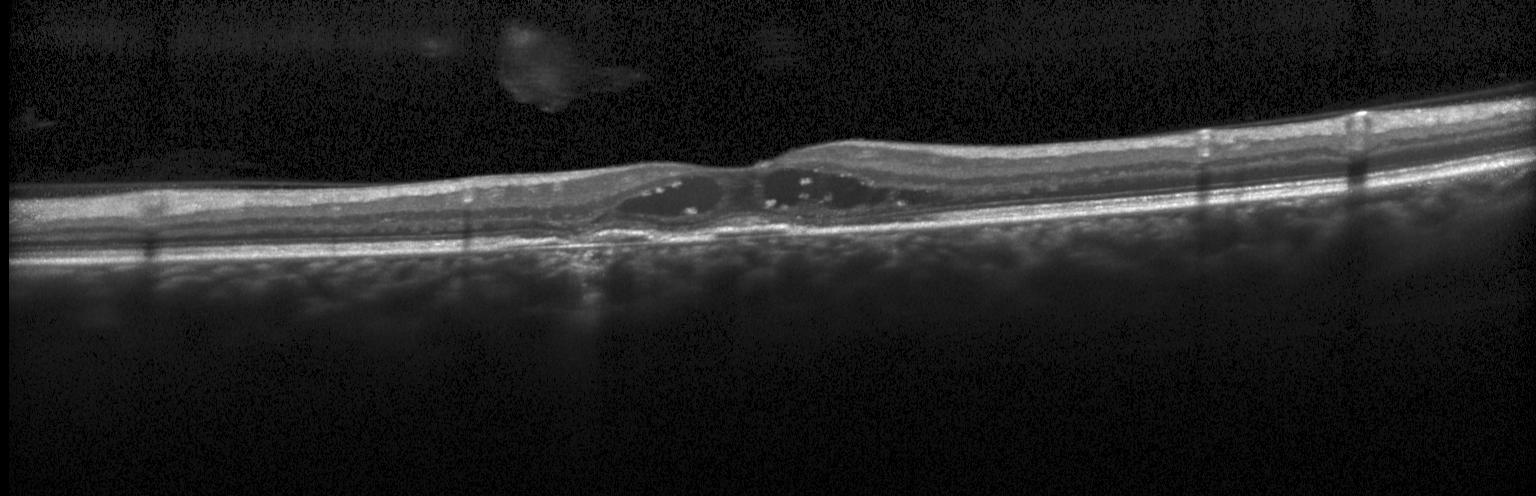 Retinal OCT cross-section showing a choroidal neovascular membrane.